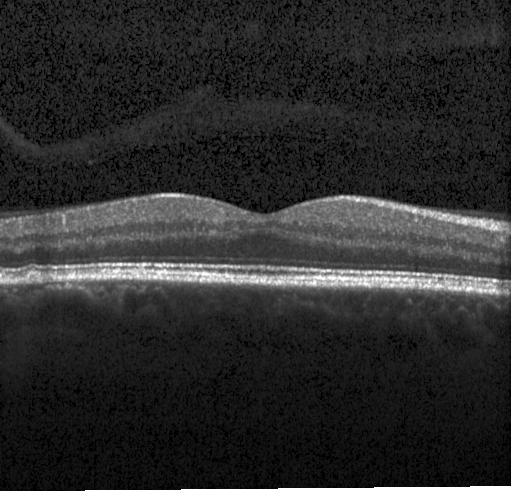

OCT scan showing drusen.